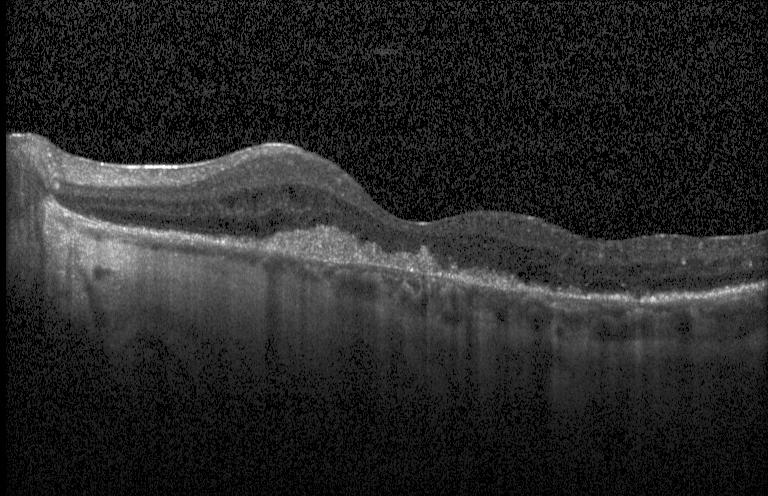

Spectral-domain optical coherence tomography · OCT B-scan
Assessment: choroidal neovascularization.